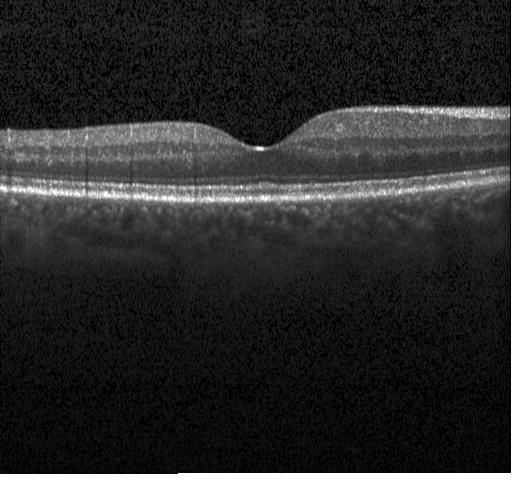

Macular OCT: no choroidal neovascularization, diabetic macular edema, or drusen.